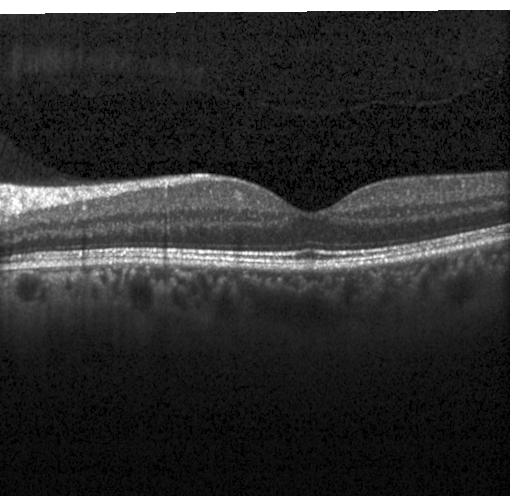

Impression: no CNV, DME, or drusen.